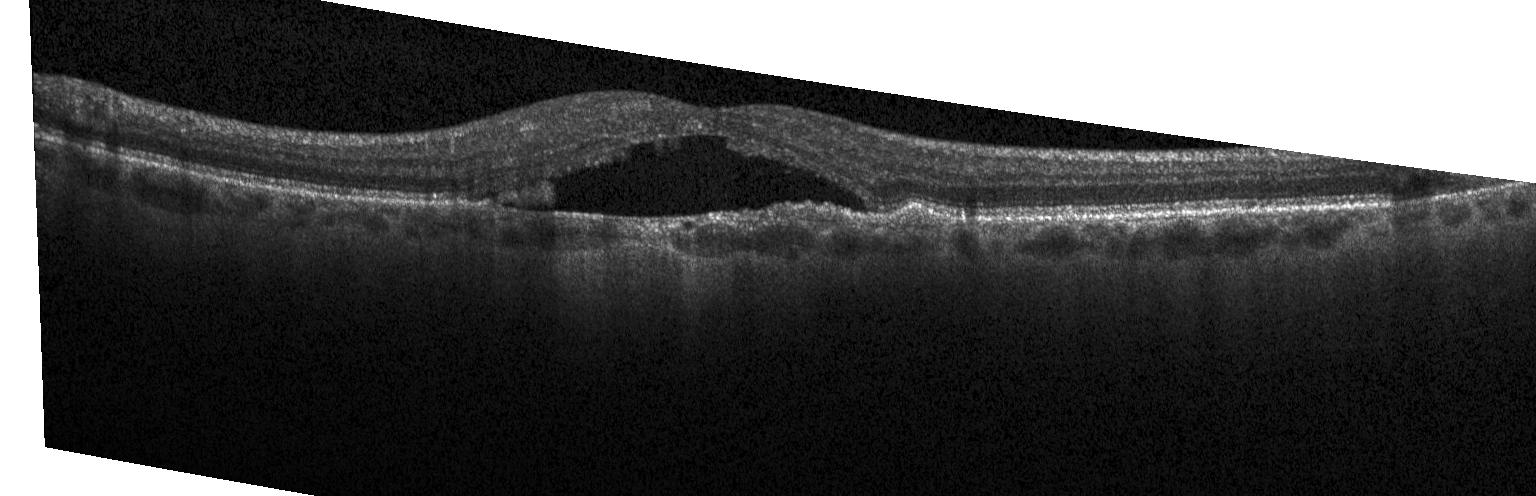
OCT B-scan. Heidelberg Spectralis — Finding: CNV.